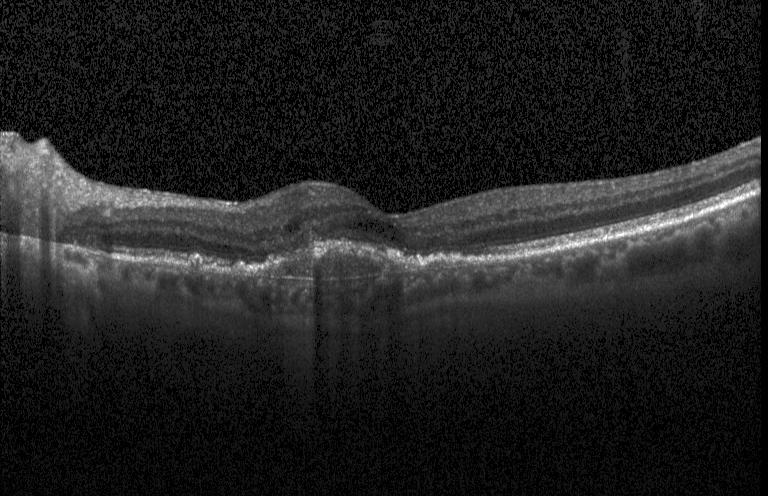

OCT B-scan showing a choroidal neovascular membrane.